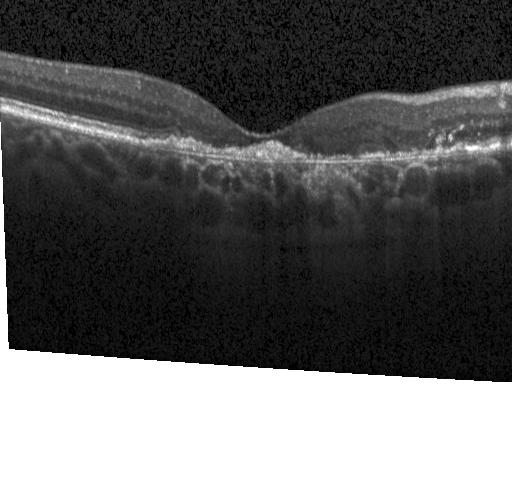

Macular scan; optical coherence tomography B-scan
Macular OCT: choroidal neovascularization (CNV).